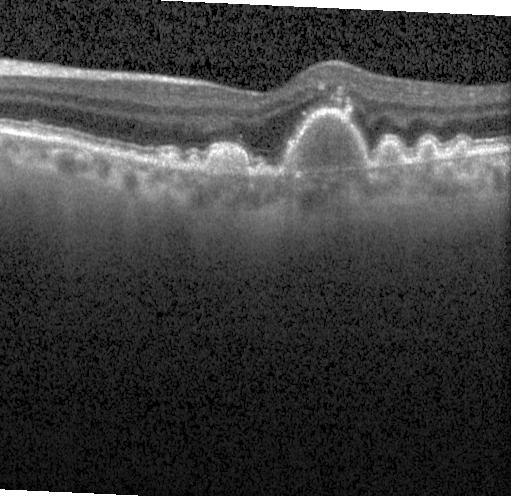

Macular OCT demonstrating multiple drusen.